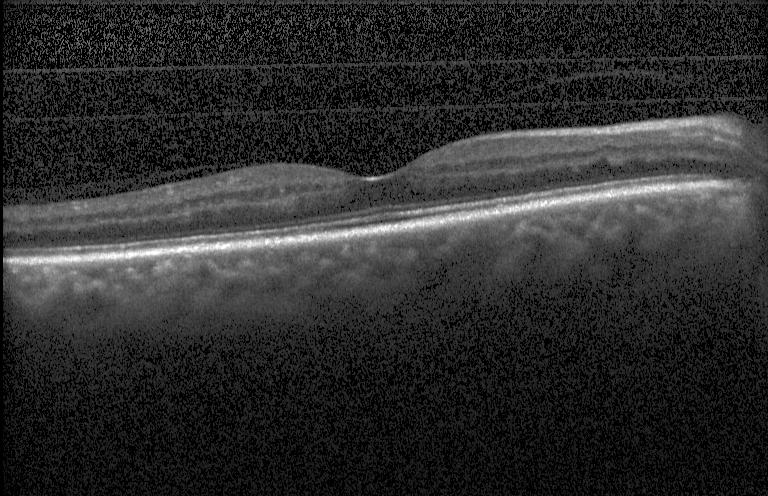
Macular OCT demonstrating no evidence of choroidal neovascularization, diabetic macular edema, or drusen.